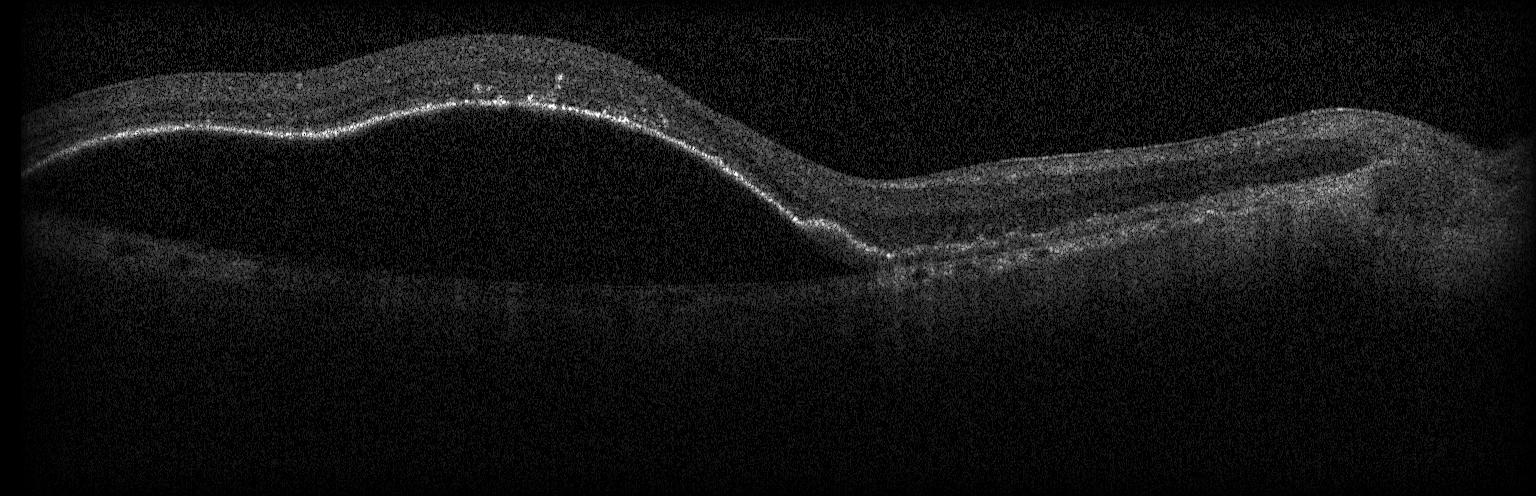 Optical coherence tomography B-scan. Finding: choroidal neovascularization (CNV).